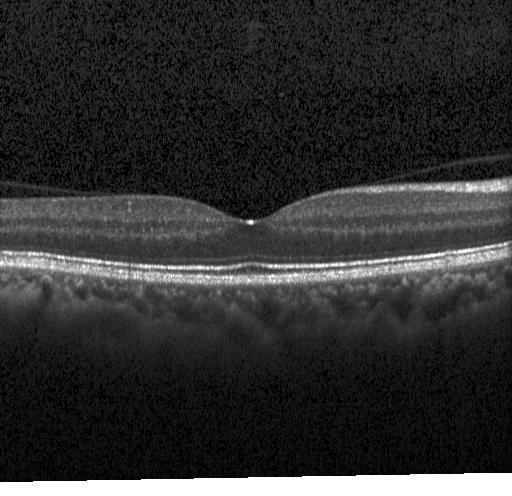

Through the macula; OCT B-scan; Heidelberg Spectralis; spectral-domain optical coherence tomography
Diagnosis: no CNV, DME, or drusen.